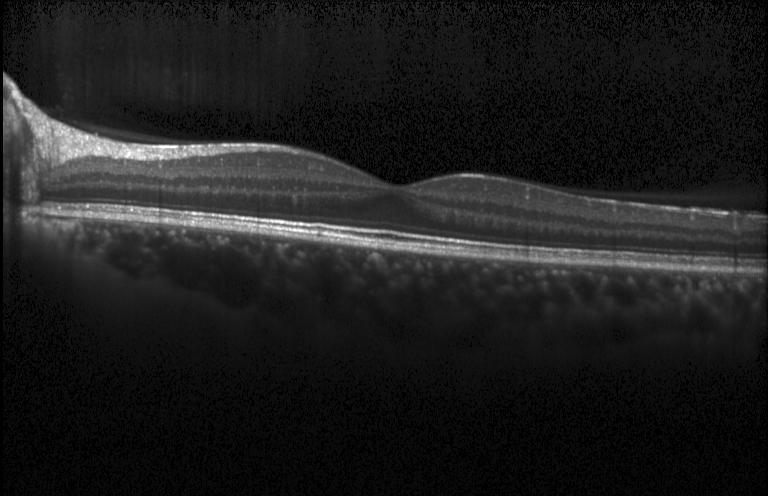
No CNV, no DME, and no drusen.